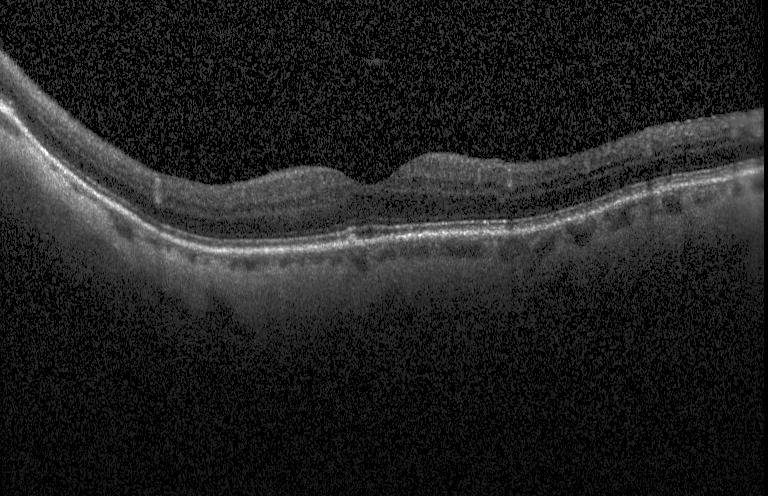

Macular OCT: multiple drusen.